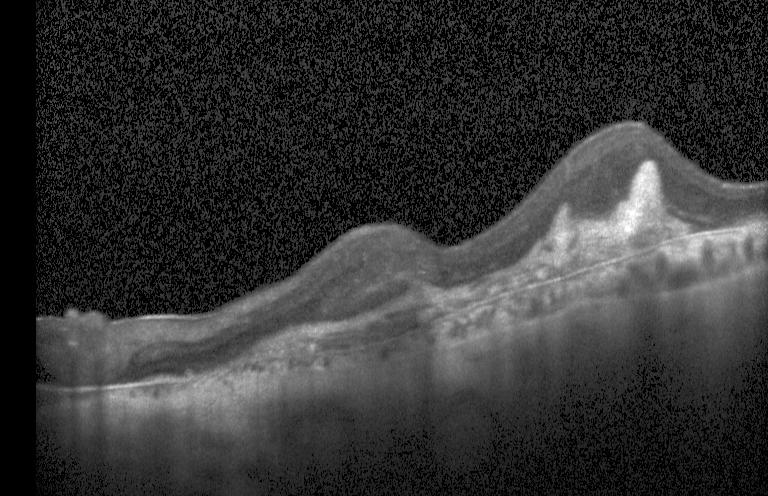 Retinal OCT cross-section. Heidelberg Spectralis OCT system. Spectral-domain optical coherence tomography. Macular OCT: choroidal neovascularization (CNV).